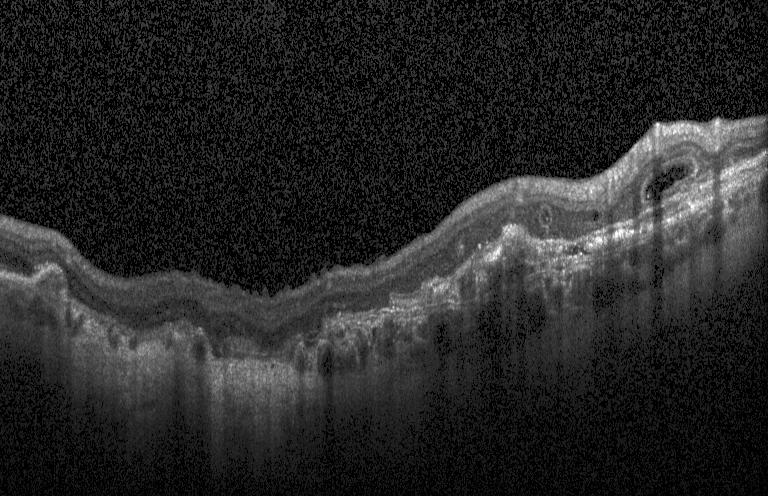 Instrument: Heidelberg Spectralis; retinal OCT cross-section.
Finding: CNV.